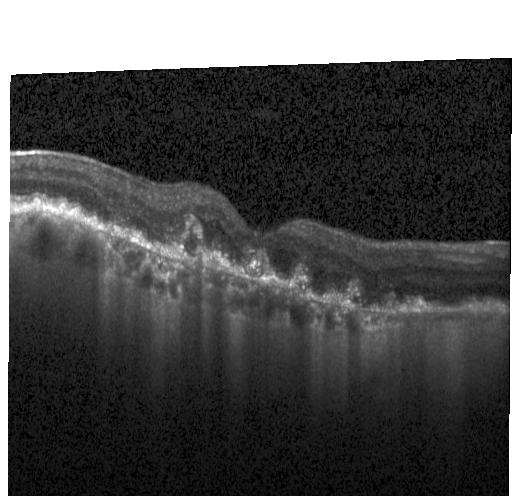 Macular OCT: a choroidal neovascular membrane.